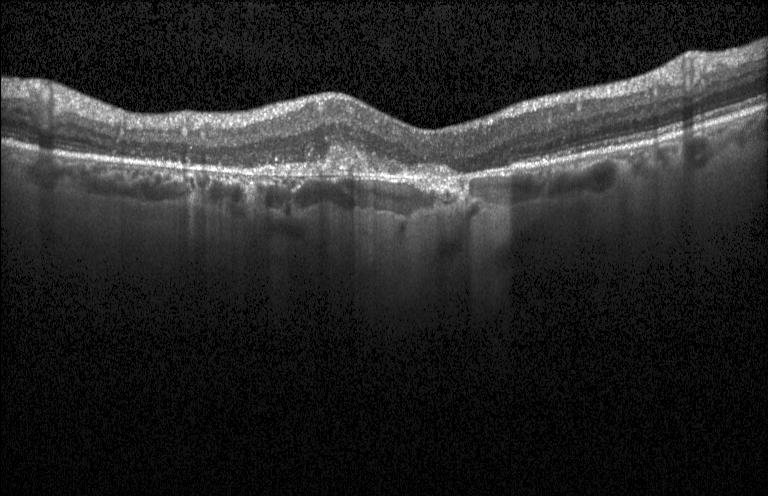 OCT B-scan showing choroidal neovascularization (CNV).